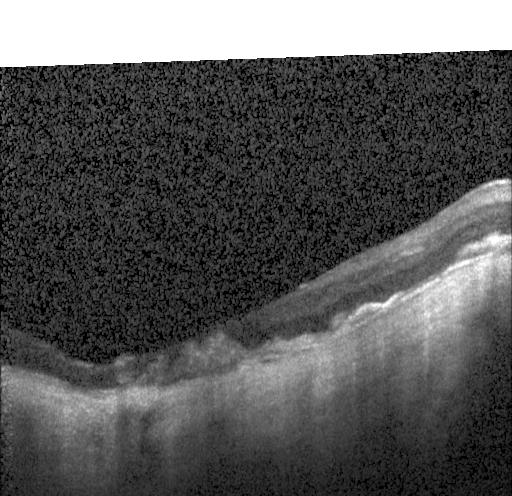
Instrument: Heidelberg Spectralis; OCT line scan.
Diagnosis: choroidal neovascularization.